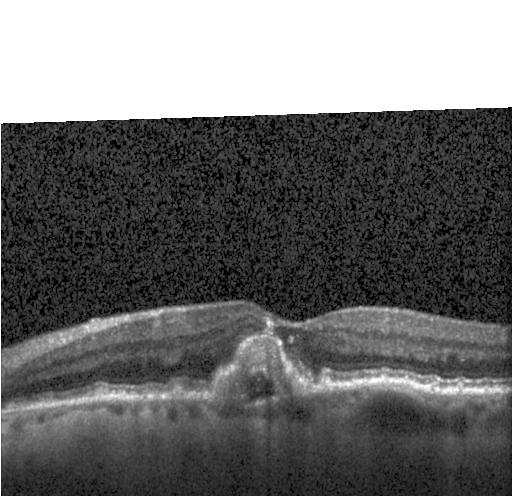

Retinal OCT B-scan · through the macula · spectral-domain OCT.
Assessment: CNV.